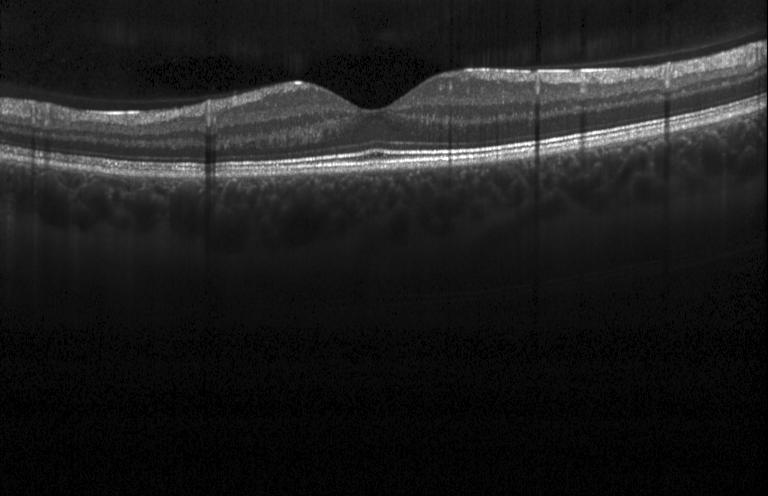
Macular OCT: no choroidal neovascularization, diabetic macular edema, or drusen.